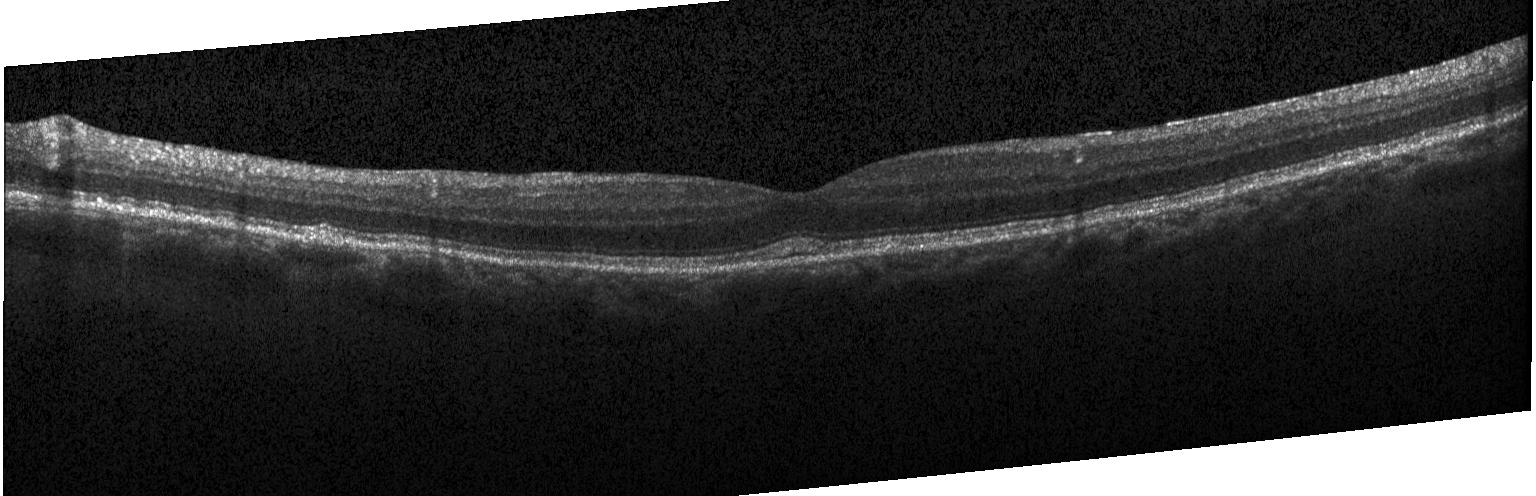

Heidelberg Spectralis; OCT line scan; SD-OCT
OCT finding: multiple drusen.